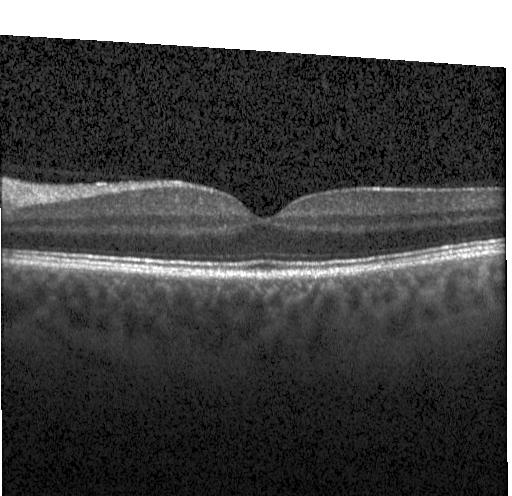 Retinal OCT B-scan, Heidelberg Spectralis, centered on the fovea. Finding: neither choroidal neovascularization, diabetic macular edema, nor drusen.